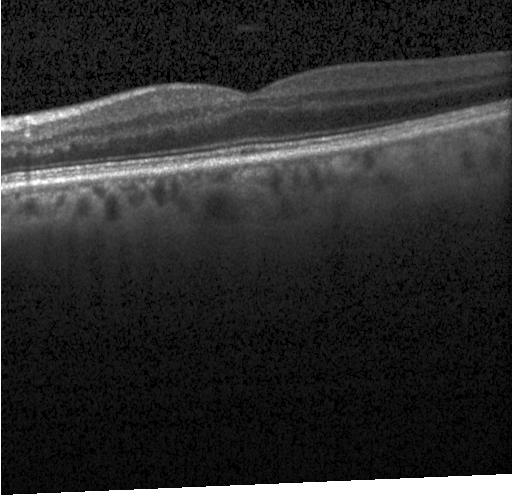
Impression: no choroidal neovascularization, no diabetic macular edema, and no drusen.